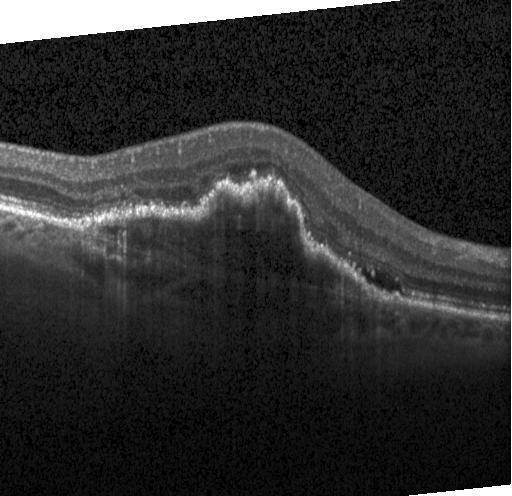
Fovea-centered · spectral-domain optical coherence tomography · optical coherence tomography scan. Impression: CNV.